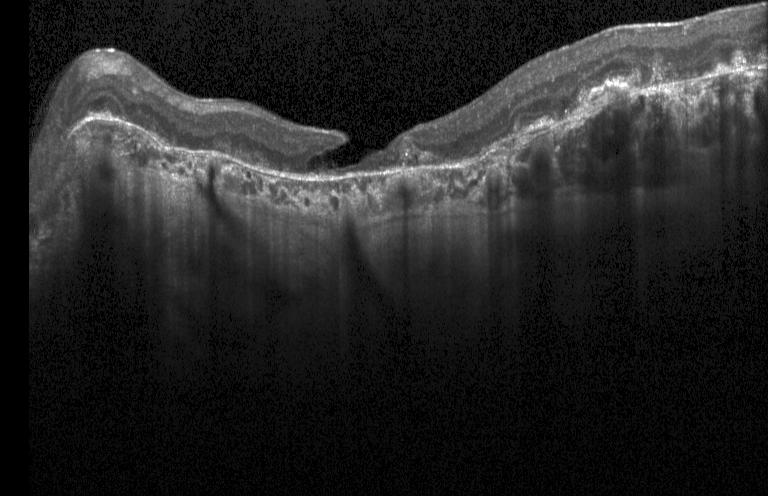 Optical coherence tomography B-scan.
Macular OCT: a choroidal neovascular membrane.